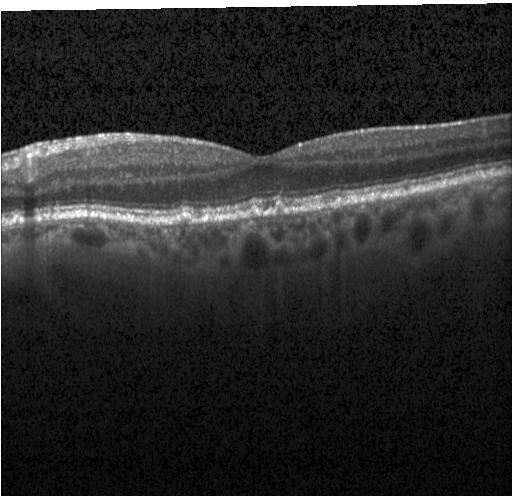 OCT scan showing sub-RPE drusenoid deposits.